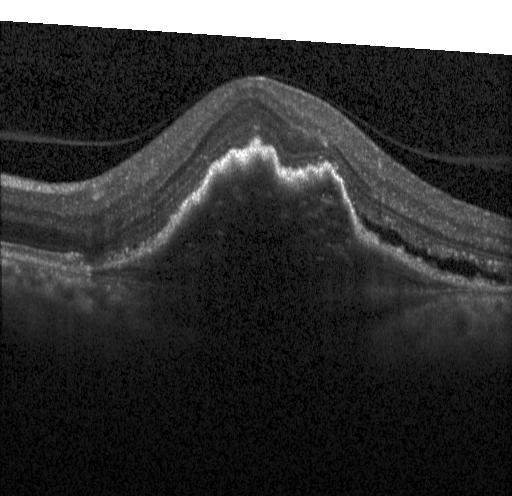

Macular OCT: a choroidal neovascular membrane.